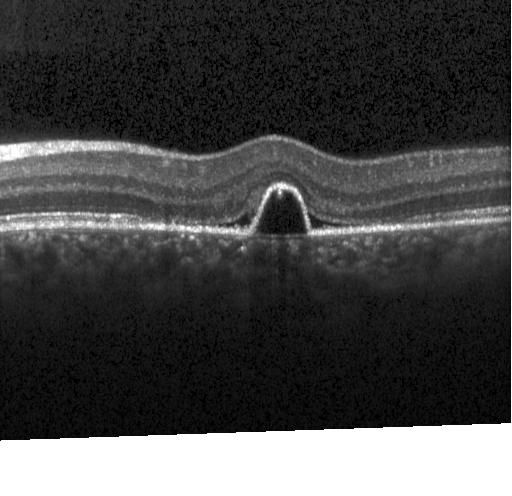
Optical coherence tomography scan, through the macula. Diagnosis: a choroidal neovascular membrane.